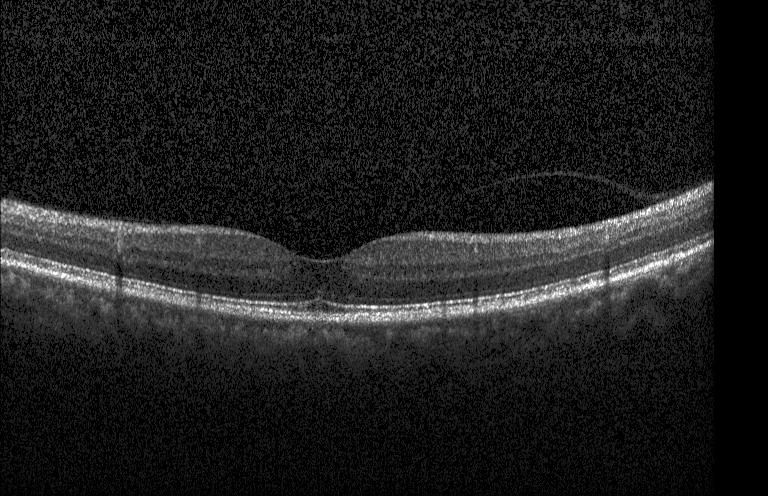

Spectral-domain optical coherence tomography, through the macula, optical coherence tomography B-scan, instrument: Heidelberg Spectralis.
Impression: no choroidal neovascularization, no diabetic macular edema, and no drusen.